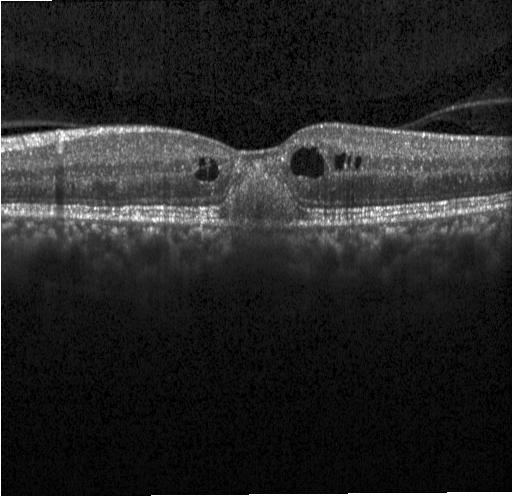

Optical coherence tomography B-scan.
Impression: a choroidal neovascular membrane.